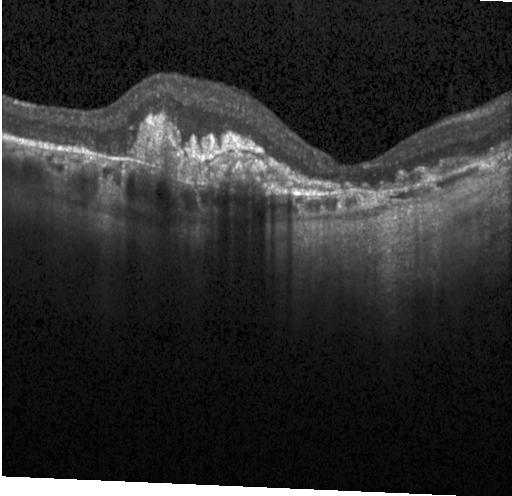
Through the macula · acquired on a Heidelberg Spectralis · optical coherence tomography B-scan.
Diagnosis: a choroidal neovascular membrane.